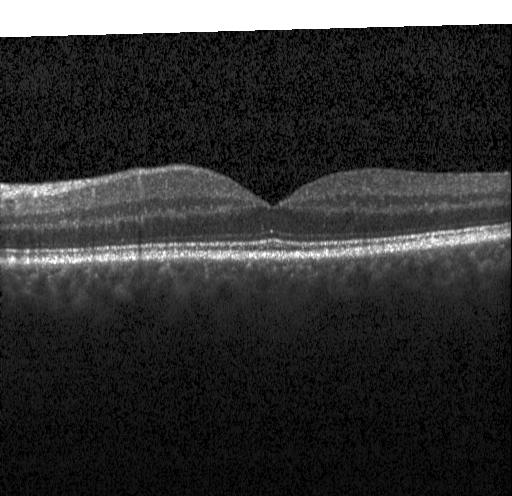

Optical coherence tomography scan.
Dx: no choroidal neovascularization, no diabetic macular edema, and no drusen.